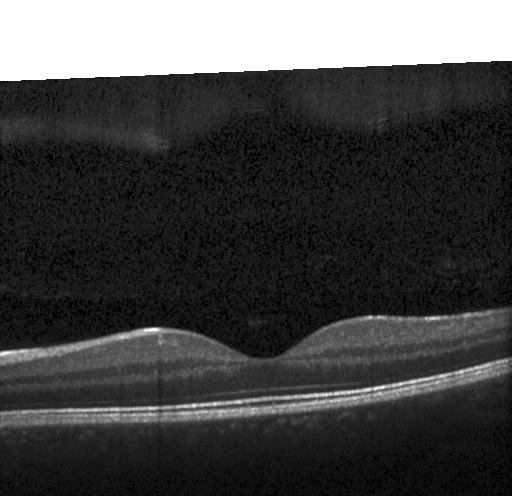
Diagnosis: no evidence of choroidal neovascularization, diabetic macular edema, or drusen.